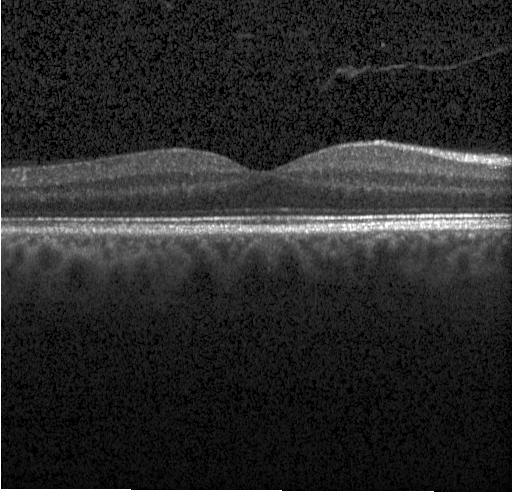 OCT B-scan — Finding: no choroidal neovascularization, no diabetic macular edema, and no drusen.